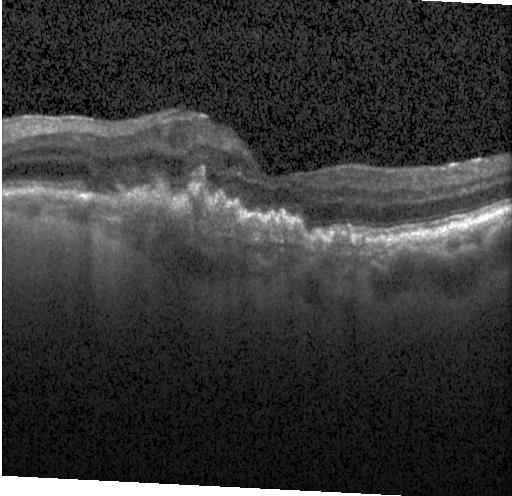
OCT line scan. Diagnosis: a choroidal neovascular membrane.